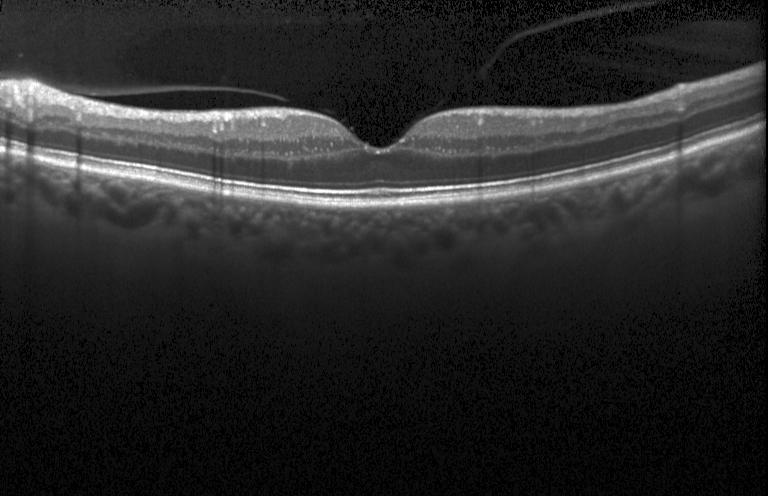

Diagnosis: neither choroidal neovascularization, diabetic macular edema, nor drusen.